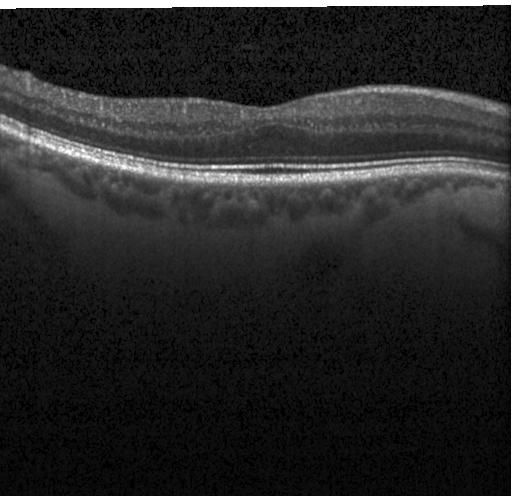

Optical coherence tomography B-scan. Diagnosis: no CNV, no DME, and no drusen.